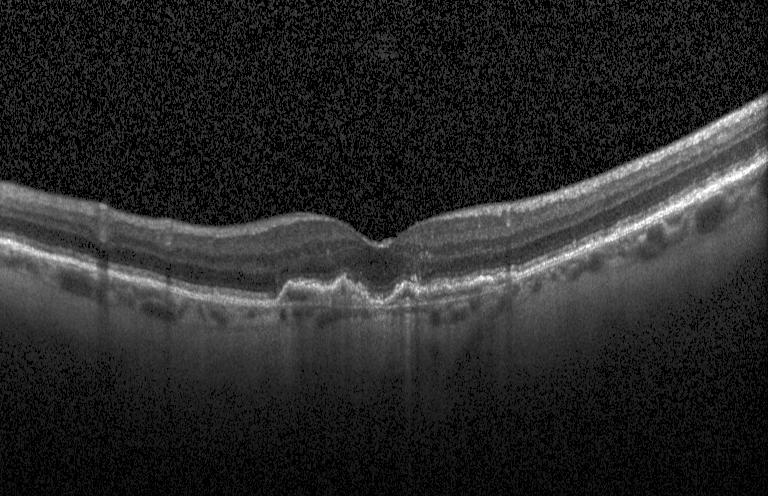 Optical coherence tomography scan, through the macula, spectral-domain optical coherence tomography.
Impression: a choroidal neovascular membrane.